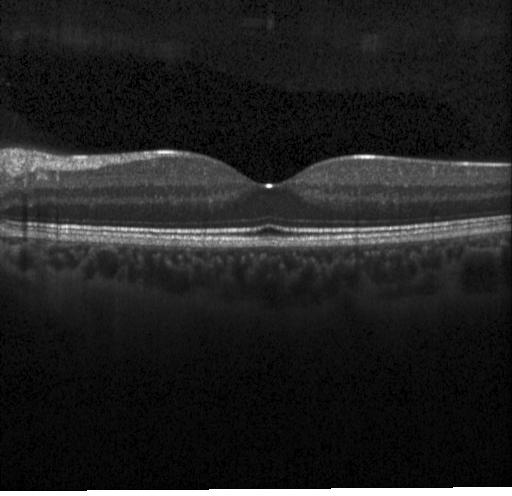
Optical coherence tomography B-scan · spectral-domain optical coherence tomography · instrument: Heidelberg Spectralis · macular scan.
Impression: no CNV, no DME, and no drusen.